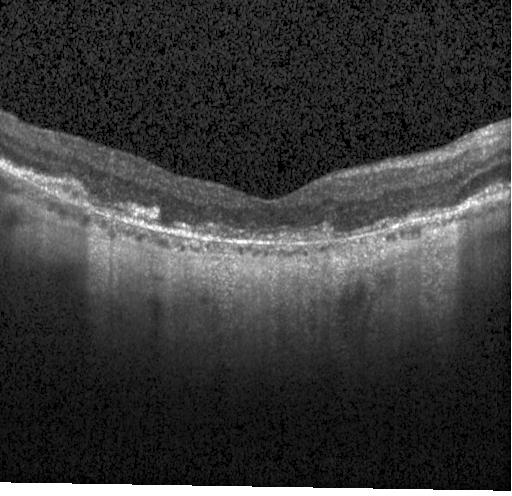 CNV.